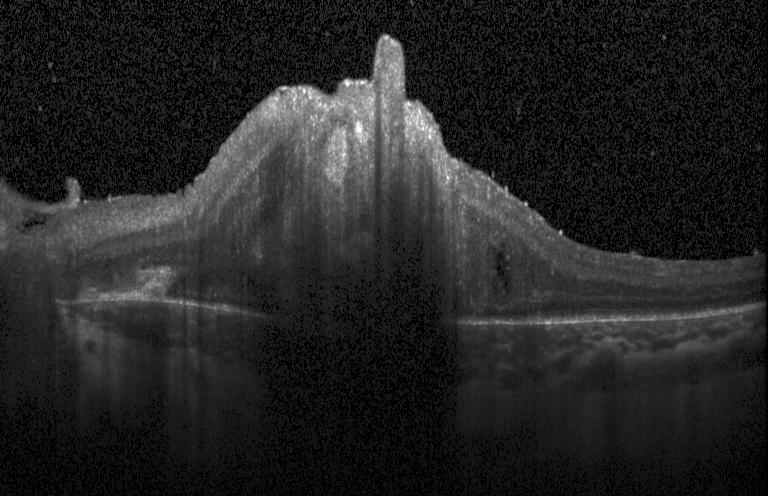
Optical coherence tomography scan, Heidelberg Spectralis, spectral-domain optical coherence tomography, macular scan. Diagnosis: a choroidal neovascular membrane.